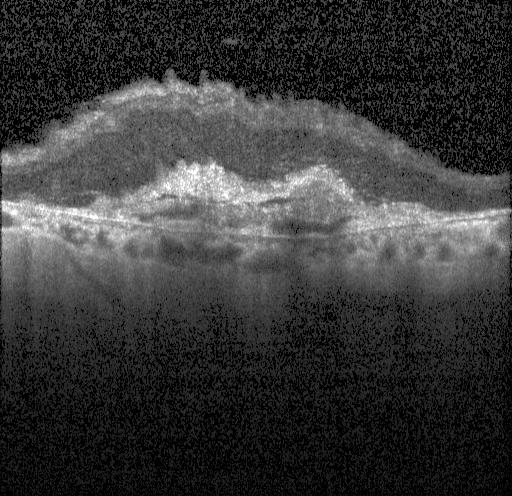

Retinal OCT cross-section.
Impression: CNV.